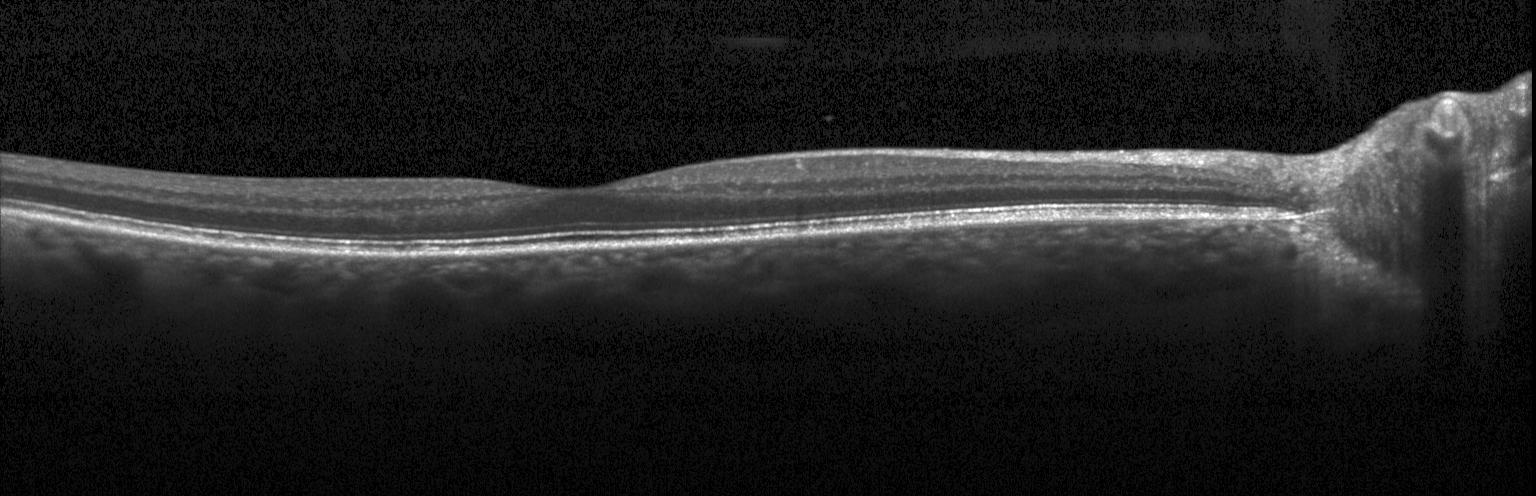 Optical coherence tomography B-scan
Macular OCT: no evidence of CNV, DME, or drusen.